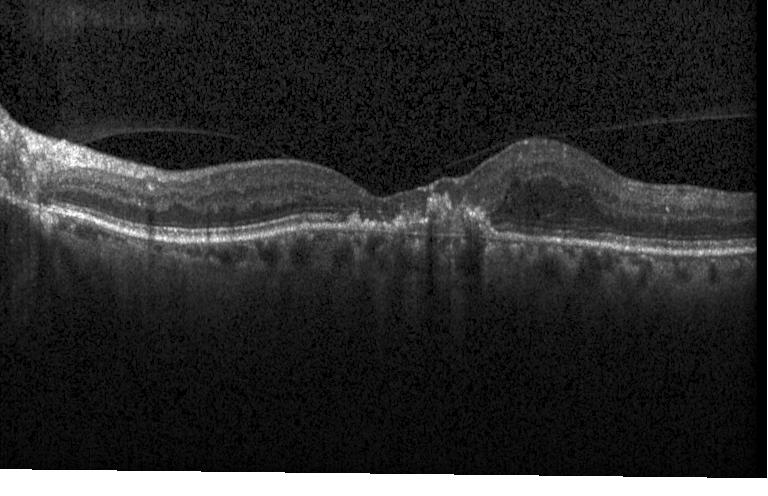 Macular OCT: choroidal neovascularization (CNV).